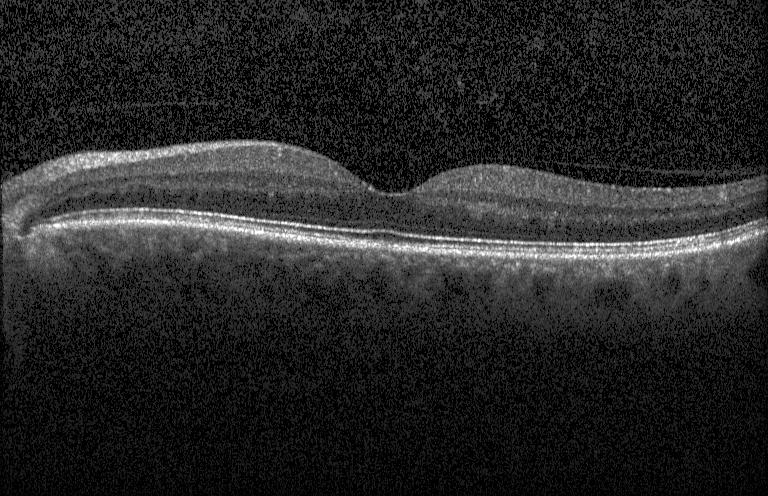 Assessment: no choroidal neovascularization, diabetic macular edema, or drusen.